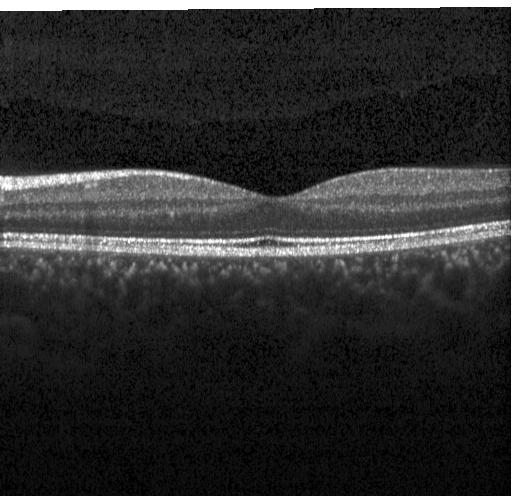 Spectral-domain OCT · fovea-centered · Heidelberg Spectralis OCT system · optical coherence tomography B-scan
Assessment: no CNV, no DME, and no drusen.